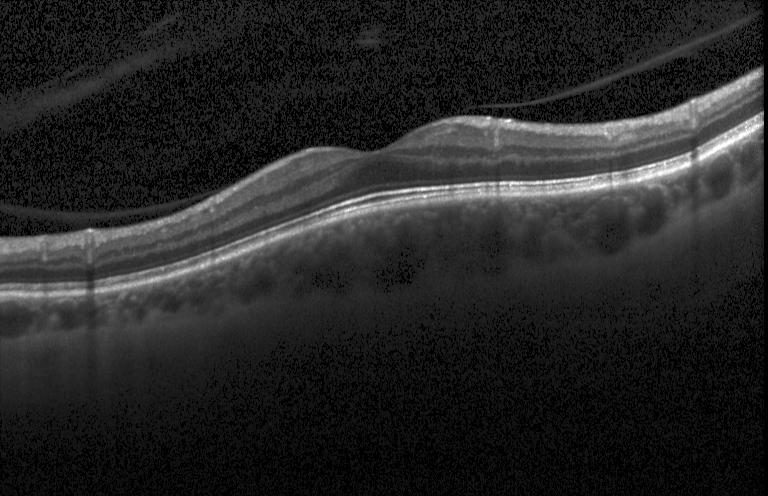

Retinal OCT cross-section showing neither choroidal neovascularization, diabetic macular edema, nor drusen.